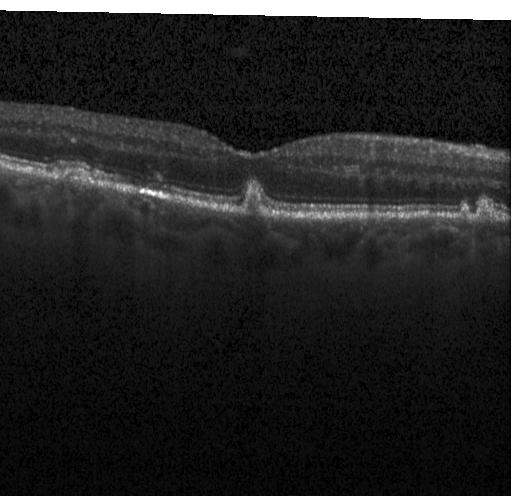 Spectral-domain OCT; macular scan; OCT B-scan.
Diagnosis: sub-RPE drusenoid deposits.